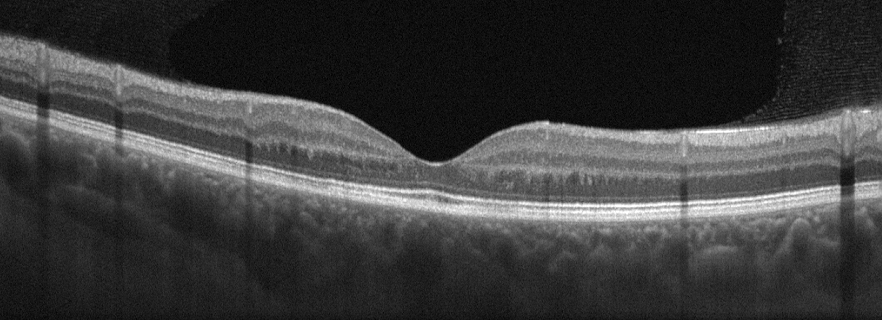 OS; retinal OCT cross-section.
Diagnosis: age-related macular degeneration (AMD).